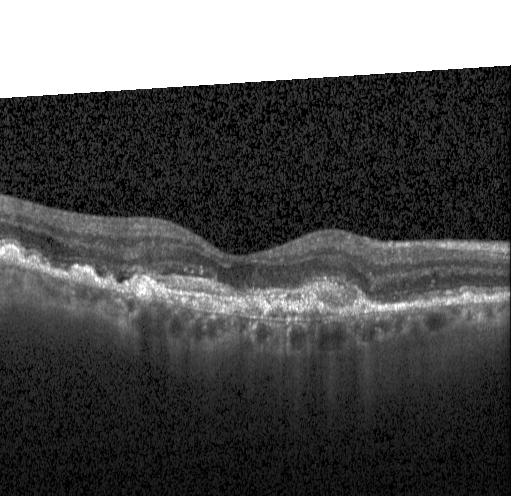 Macular OCT demonstrating CNV.